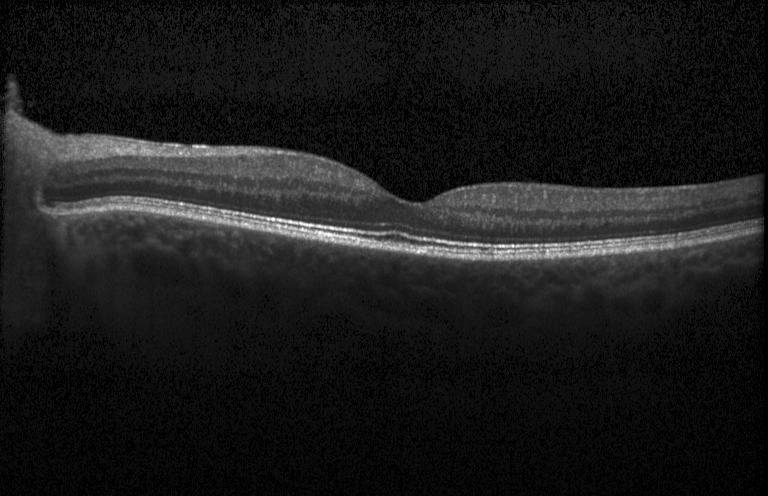
OCT finding: no choroidal neovascularization, no diabetic macular edema, and no drusen.